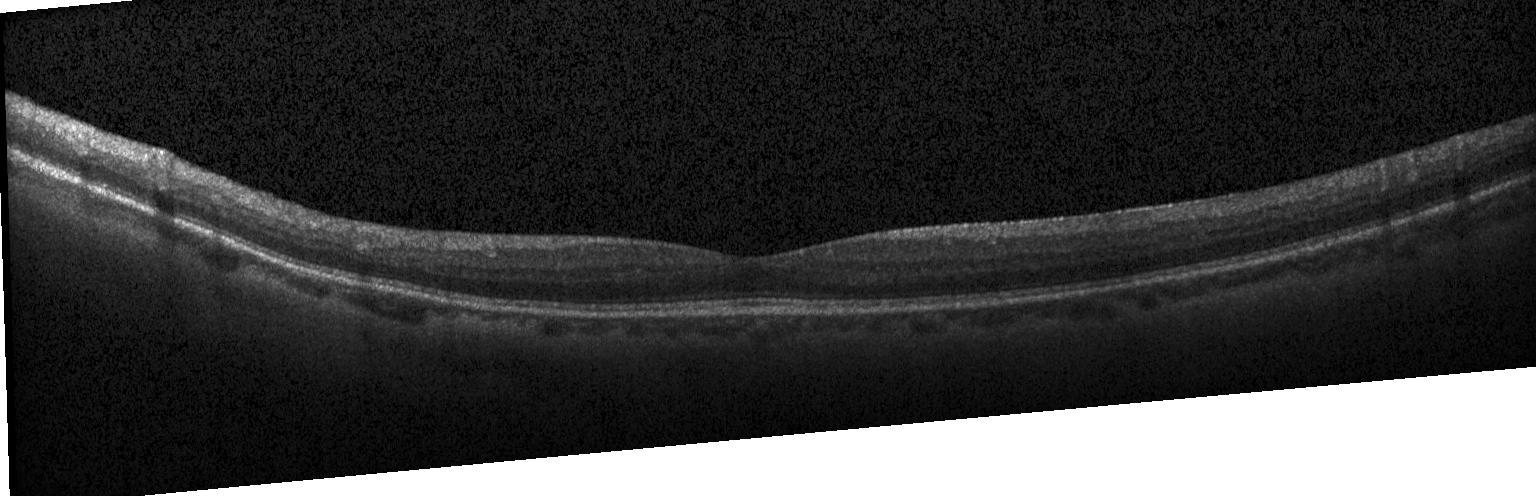 Optical coherence tomography scan. Impression: no evidence of choroidal neovascularization, diabetic macular edema, or drusen.